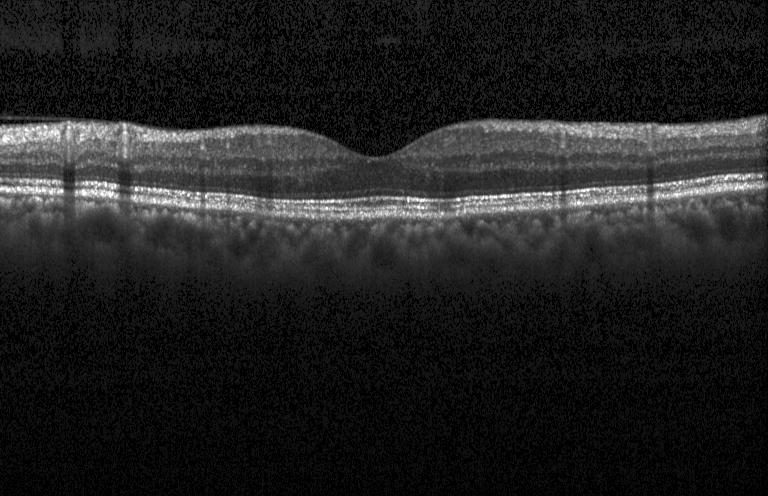

Spectral-domain optical coherence tomography · retinal OCT B-scan.
Macular OCT: no choroidal neovascularization, no diabetic macular edema, and no drusen.